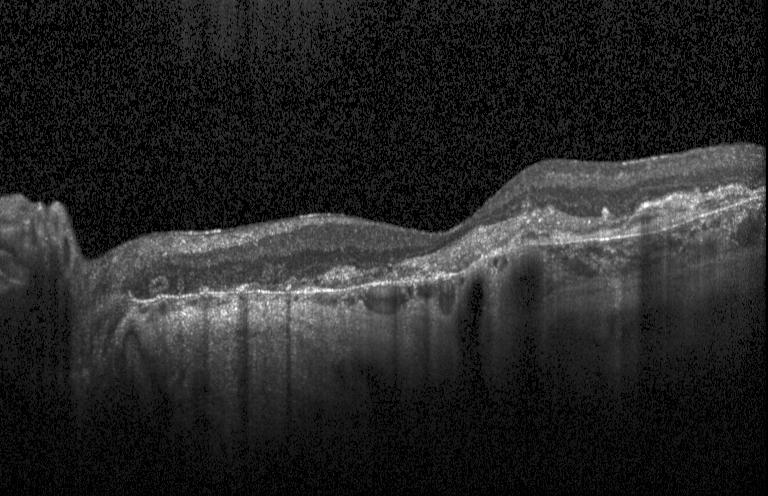
Fovea-centered, spectral-domain optical coherence tomography, optical coherence tomography scan
Dx: a choroidal neovascular membrane.